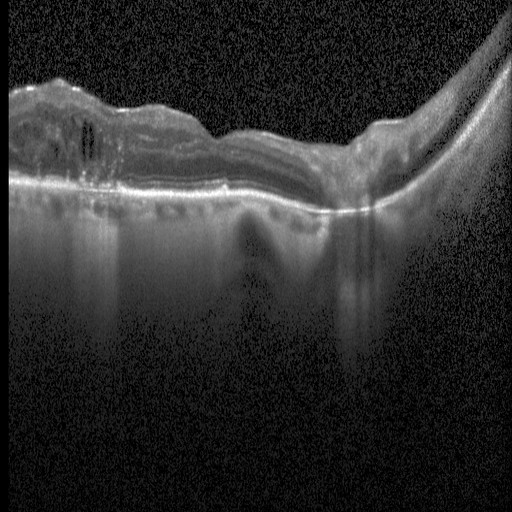 Diabetic macular edema (DME).